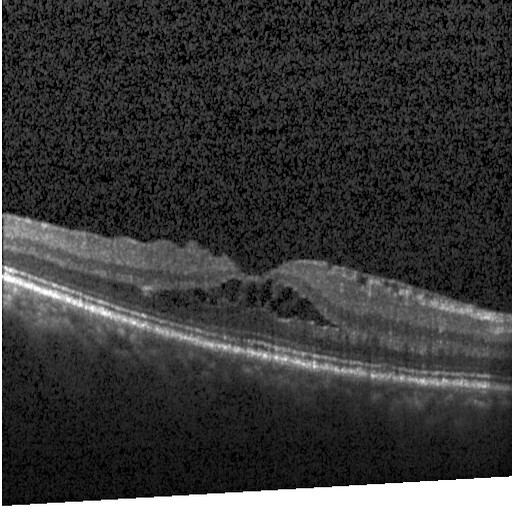
Spectral-domain optical coherence tomography. Acquired on a Heidelberg Spectralis. Retinal OCT cross-section. Diagnosis: diabetic macular edema (DME).